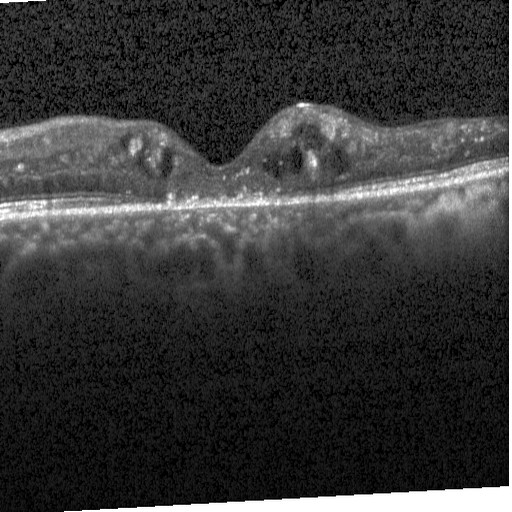 Retinal OCT cross-section
Diagnosis: DME.